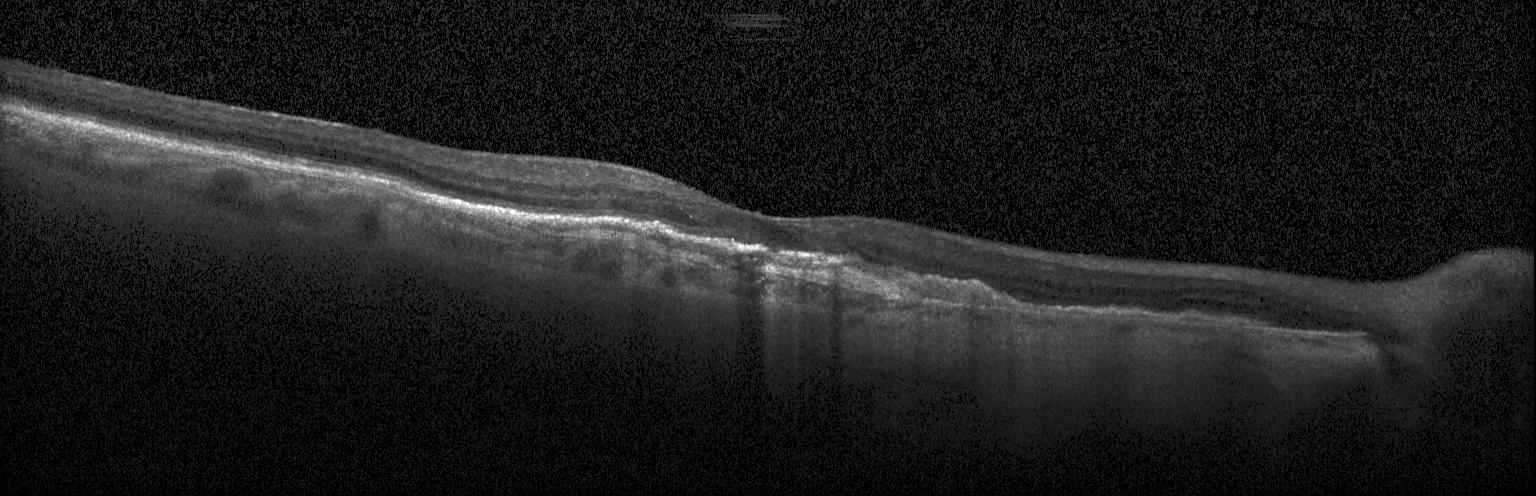

OCT B-scan — CNV.